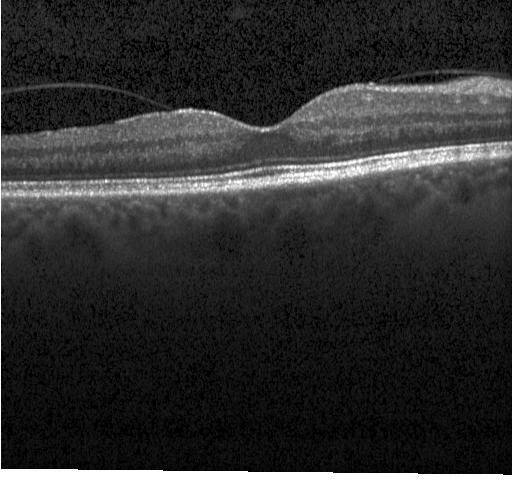
Spectral-domain OCT; macular scan; acquired on a Heidelberg Spectralis; retinal OCT B-scan
Dx: neither CNV, DME, nor drusen.